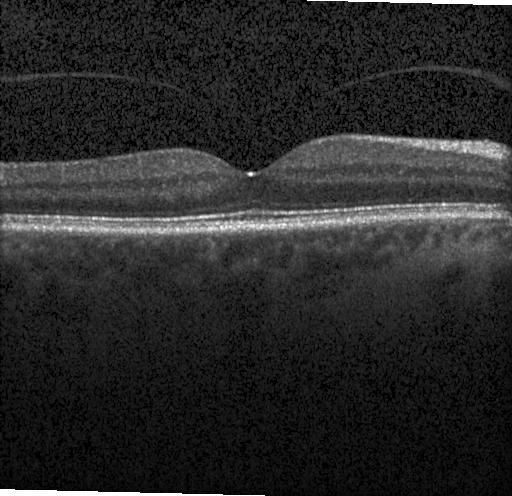
OCT B-scan, Heidelberg Spectralis OCT system, fovea-centered, spectral-domain optical coherence tomography — Diagnosis: no CNV, DME, or drusen.